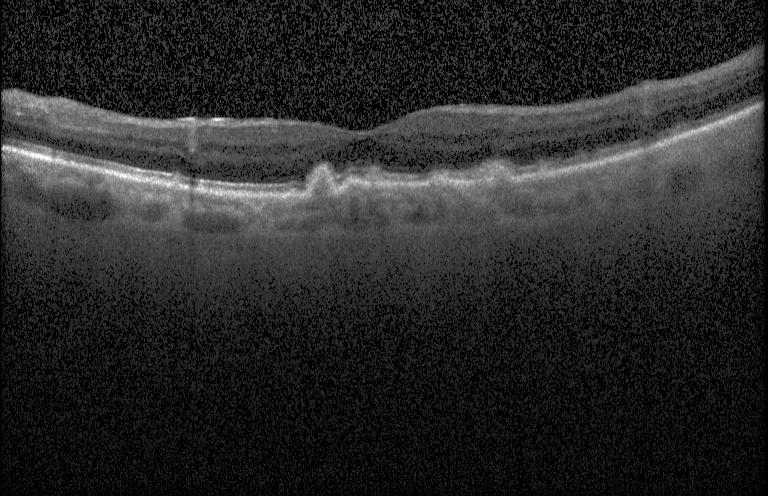 Spectral-domain OCT B-scan: drusen.